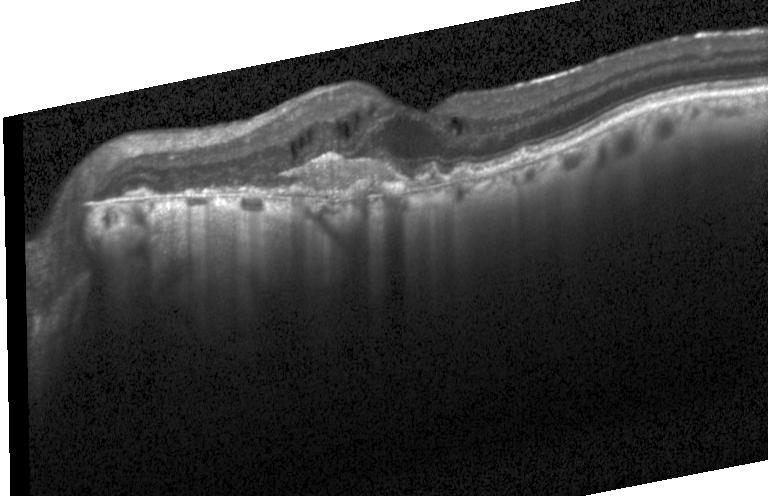
OCT line scan.
This B-scan demonstrates CNV.